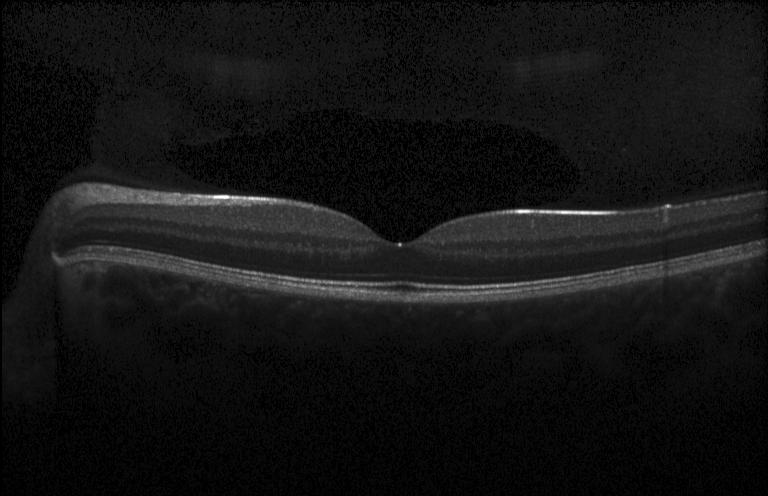
Macular scan · Heidelberg Spectralis OCT system · retinal OCT cross-section — Finding: no choroidal neovascularization, diabetic macular edema, or drusen.